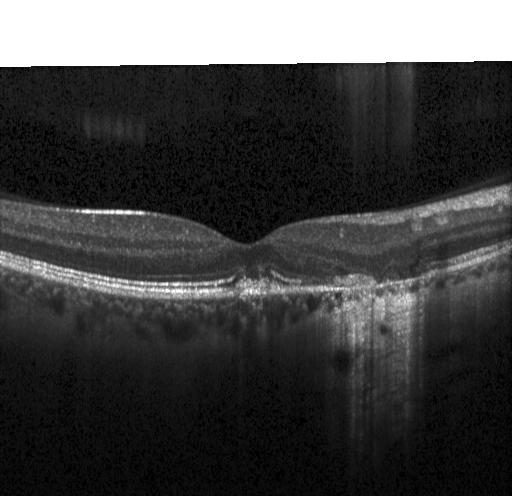
Retinal OCT cross-section · spectral-domain optical coherence tomography. Impression: CNV.